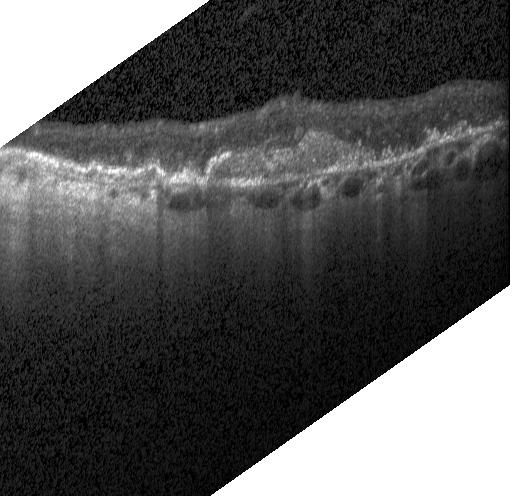
OCT line scan. Acquired on a Heidelberg Spectralis.
Dx: choroidal neovascularization.